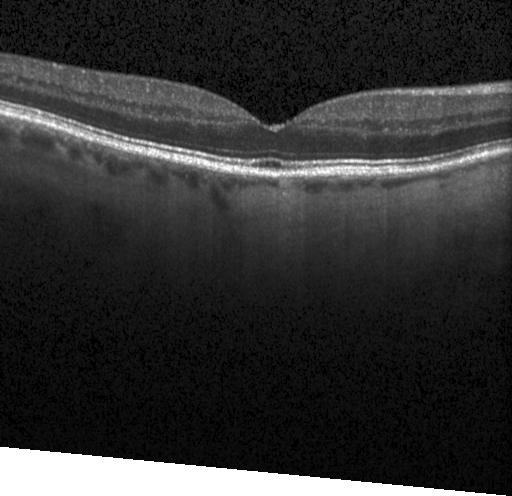 Centered on the fovea · optical coherence tomography scan.
Impression: neither CNV, DME, nor drusen.